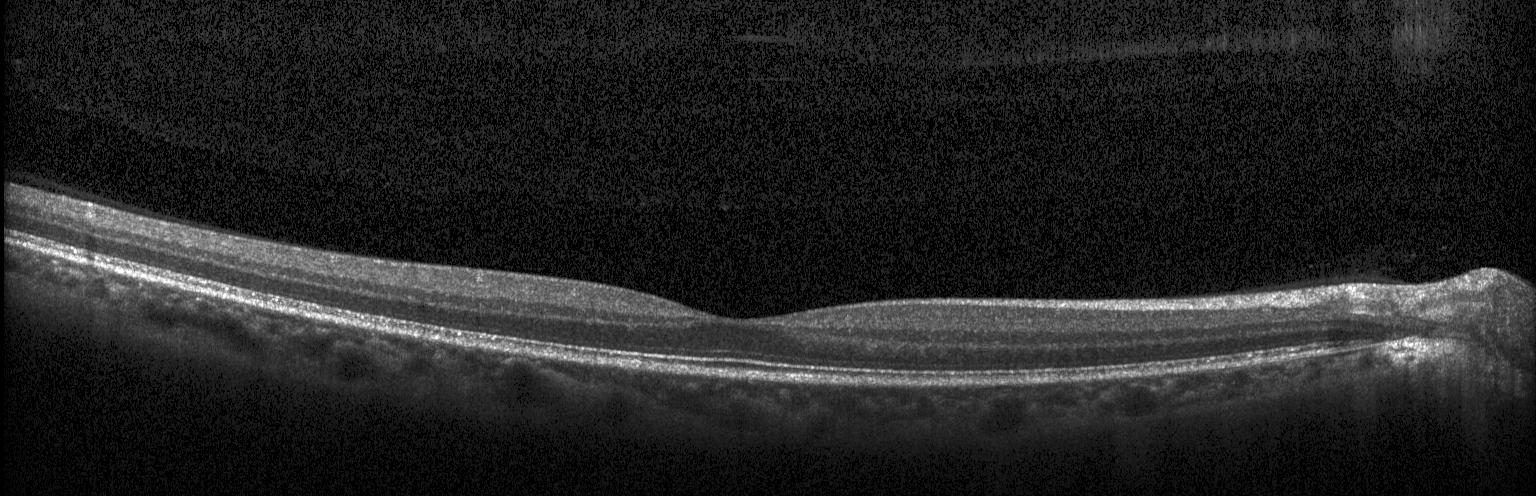 Centered on the fovea, instrument: Heidelberg Spectralis, OCT line scan, spectral-domain OCT. Diagnosis: no evidence of choroidal neovascularization, diabetic macular edema, or drusen.